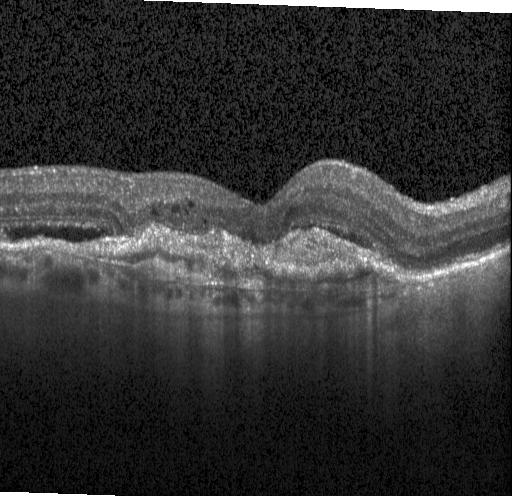

Spectral-domain optical coherence tomography, OCT line scan, through the macula — Macular OCT: a choroidal neovascular membrane.